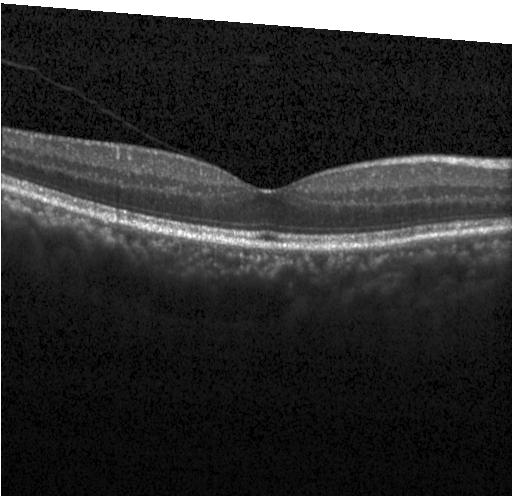 OCT B-scan.
Diagnosis: neither choroidal neovascularization, diabetic macular edema, nor drusen.